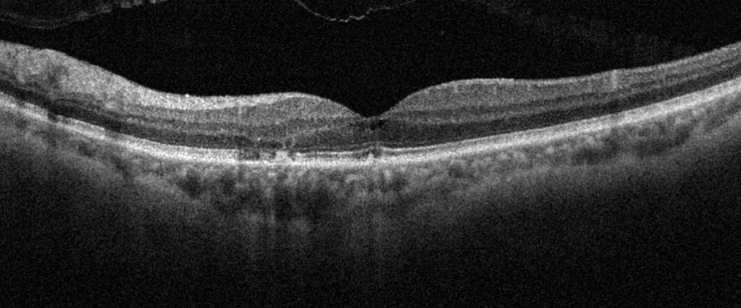 Retinal OCT B-scan
This B-scan demonstrates age-related macular degeneration.